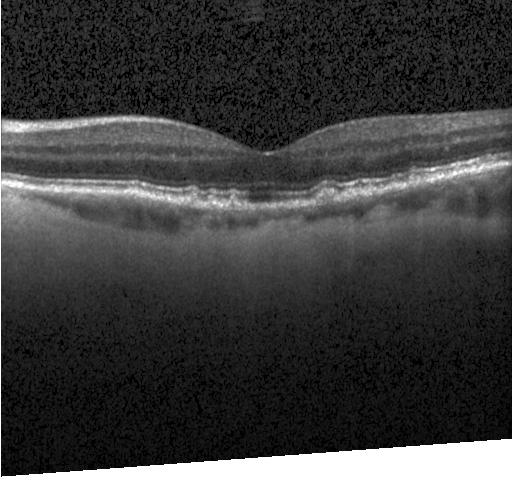
Spectral-domain OCT; retinal OCT B-scan — This B-scan demonstrates drusen.